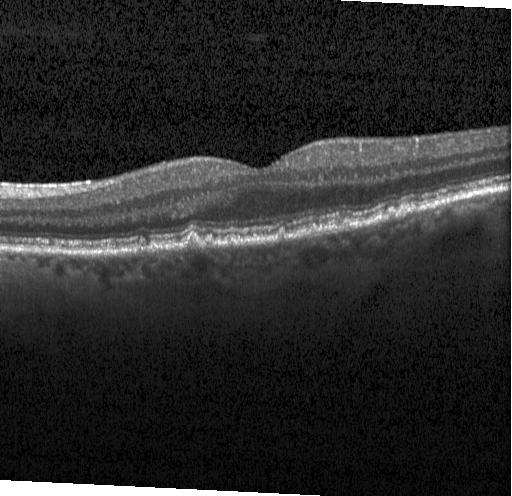
Heidelberg Spectralis OCT system. Optical coherence tomography B-scan — Finding: drusen.